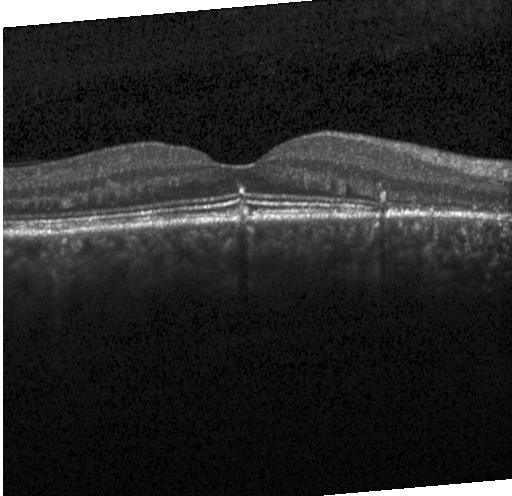

Acquired on a Heidelberg Spectralis · retinal OCT B-scan.
Dx: drusen.